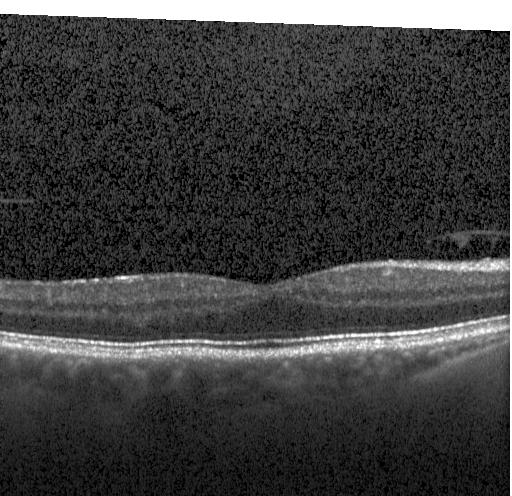
Assessment: no evidence of choroidal neovascularization, diabetic macular edema, or drusen.